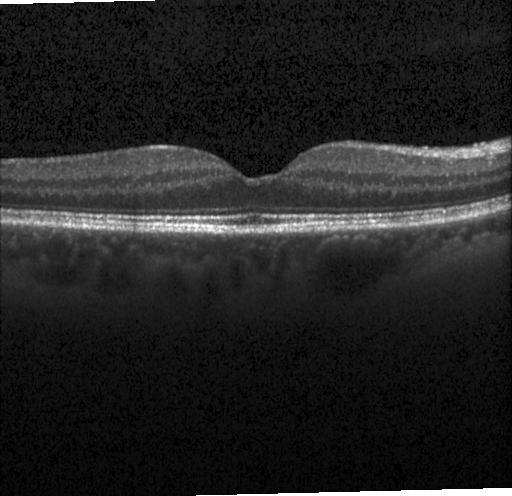 Diagnosis: neither CNV, DME, nor drusen.